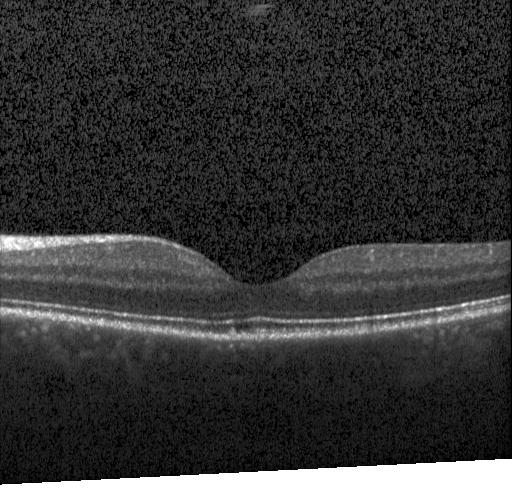

No choroidal neovascularization, no diabetic macular edema, and no drusen.